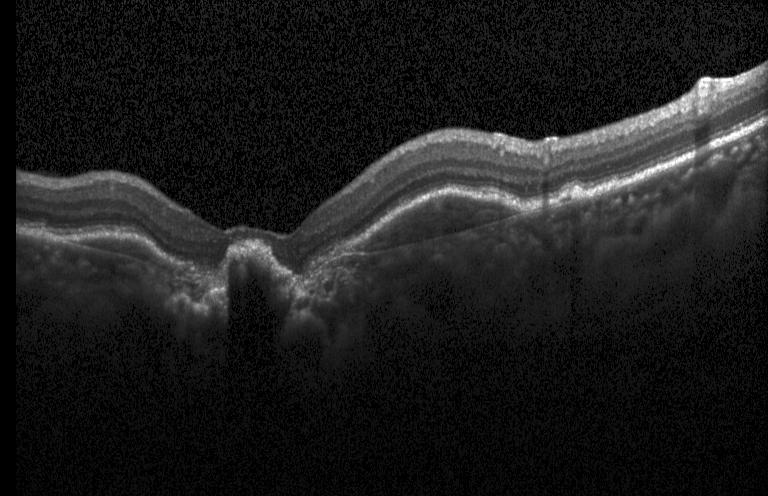

OCT scan showing a choroidal neovascular membrane.